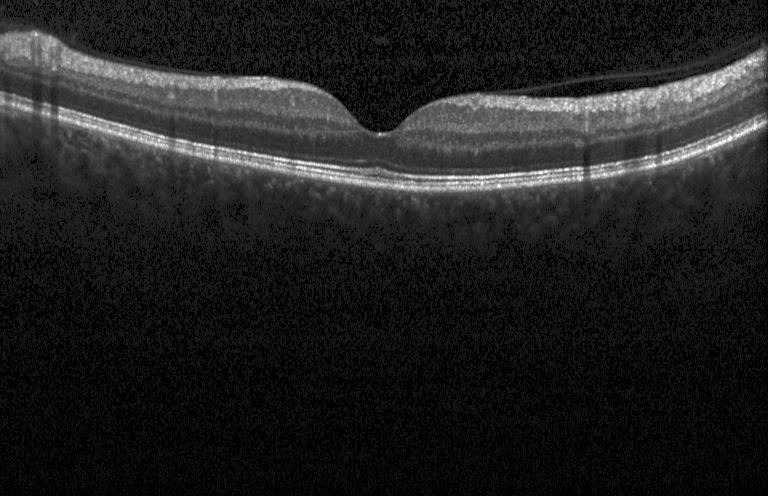
Optical coherence tomography scan · macular scan.
OCT finding: no choroidal neovascularization, diabetic macular edema, or drusen.